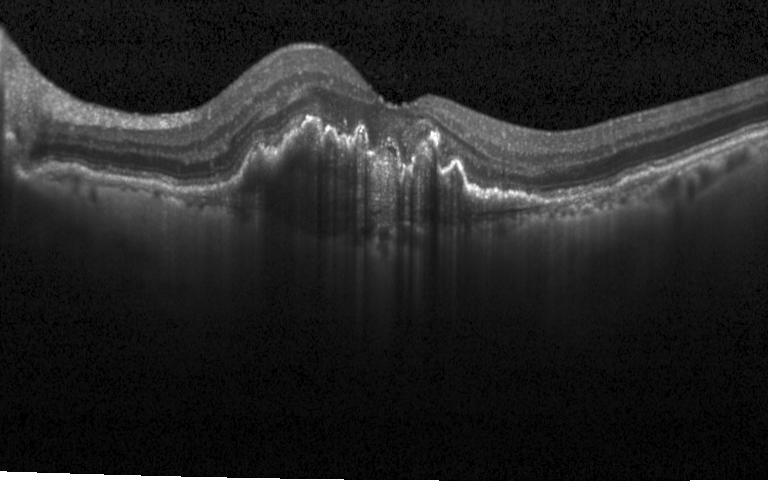

Retinal OCT cross-section. Centered on the fovea. Spectral-domain OCT. Heidelberg Spectralis OCT system.
OCT finding: a choroidal neovascular membrane.